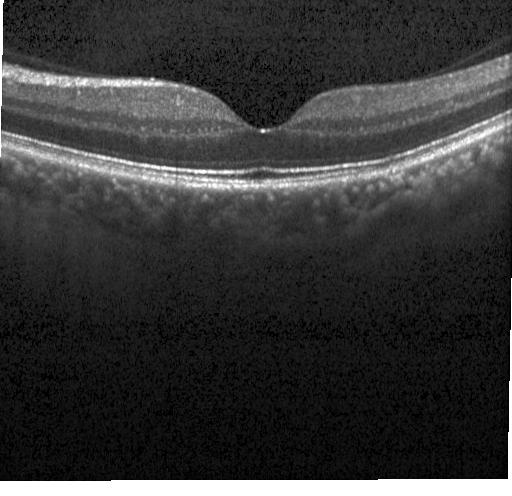

Dx: no CNV, DME, or drusen.